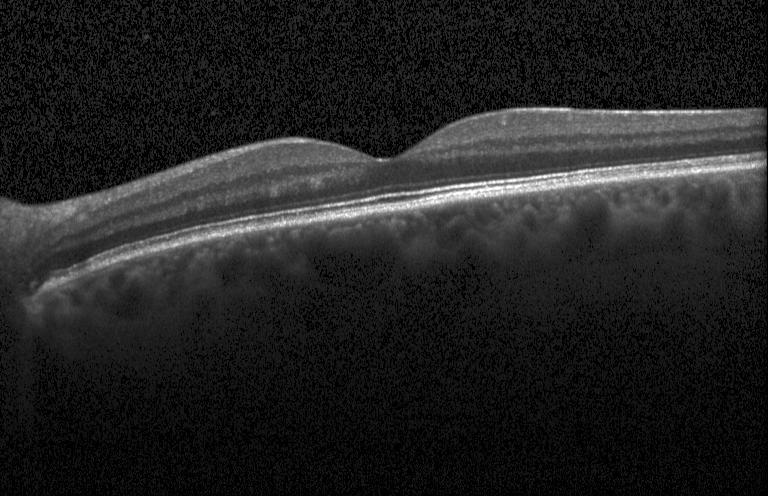
This B-scan demonstrates no choroidal neovascularization, no diabetic macular edema, and no drusen.